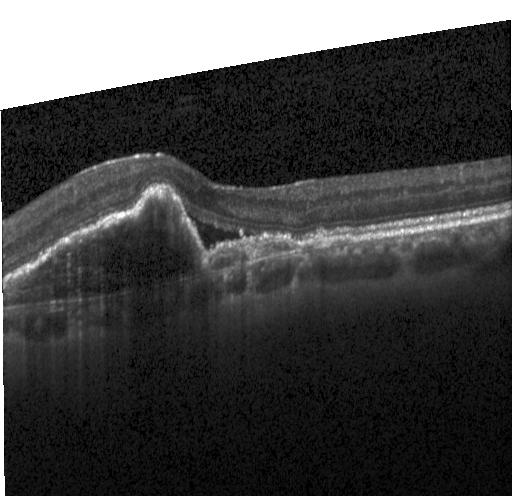 Retinal OCT cross-section; through the macula; acquired on a Heidelberg Spectralis — Impression: a choroidal neovascular membrane.